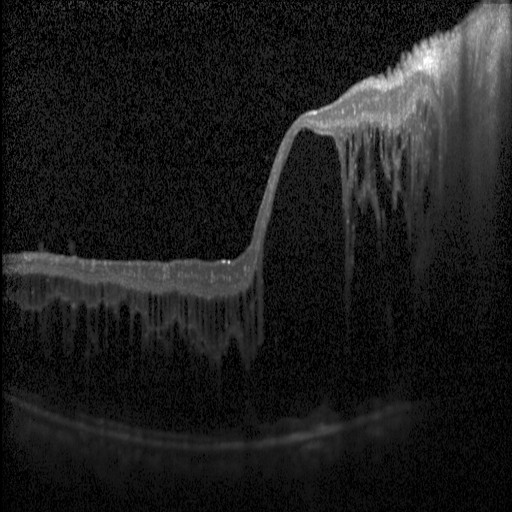
Macular OCT: diabetic macular edema (DME).